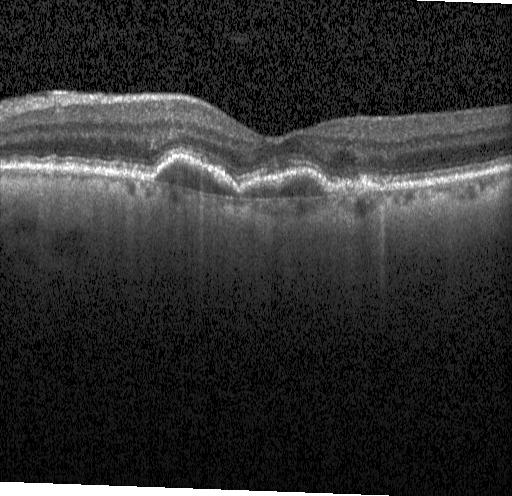

Retinal OCT cross-section; spectral-domain OCT. Diagnosis: CNV.